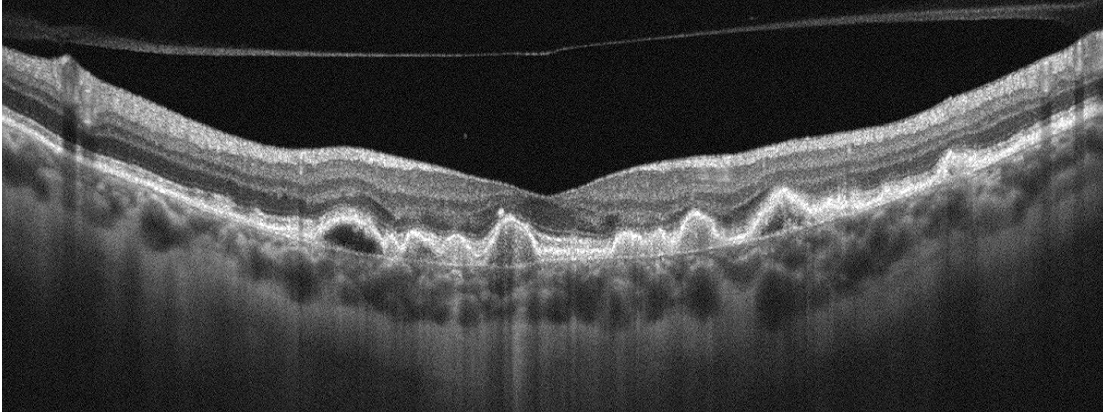

Optovue Avanti RTVue XR · retinal OCT cross-section. Finding: age-related macular degeneration.